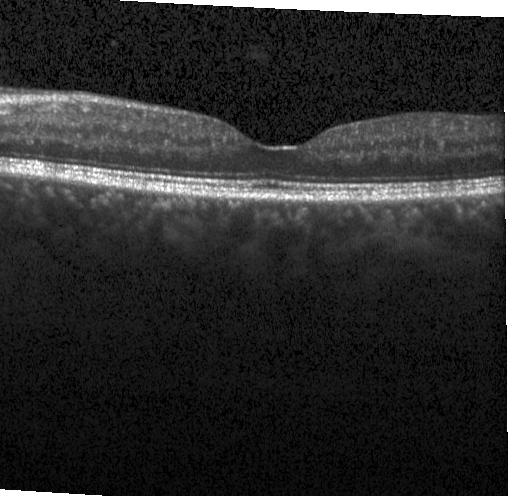

Horizontal scan through the fovea, spectral-domain optical coherence tomography, OCT B-scan
Assessment: no CNV, DME, or drusen.